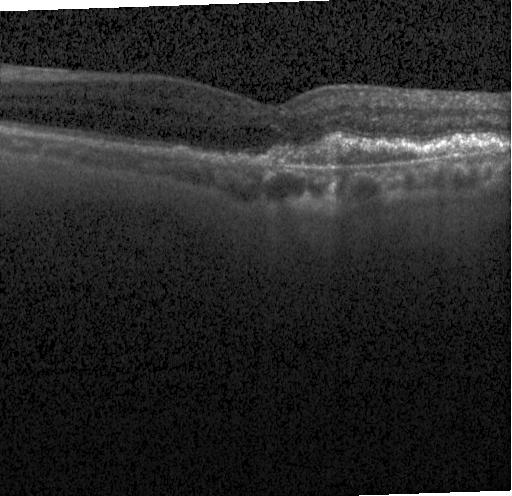 Optical coherence tomography B-scan; fovea-centered.
Choroidal neovascularization.